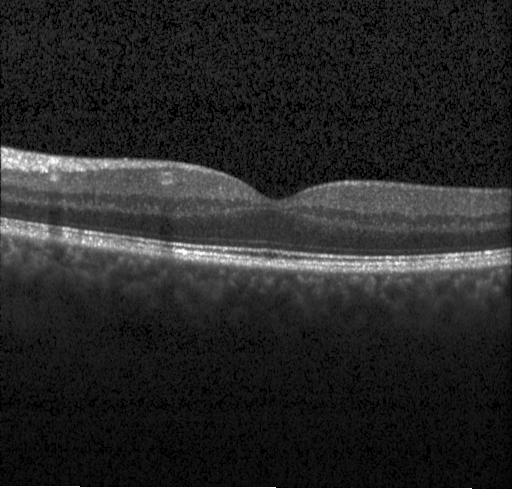 Instrument: Heidelberg Spectralis. Macular scan. OCT line scan. SD-OCT. Impression: no choroidal neovascularization, no diabetic macular edema, and no drusen.